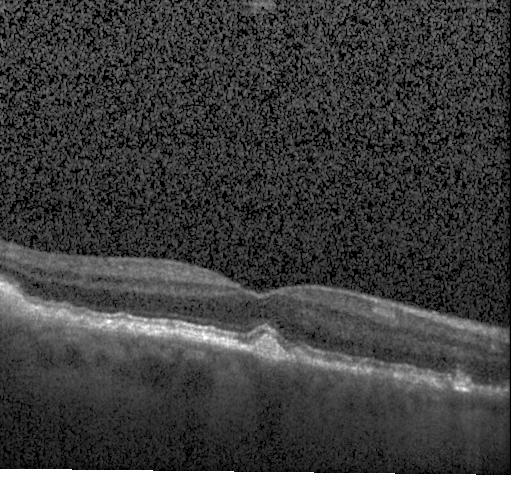
Dx: multiple drusen.